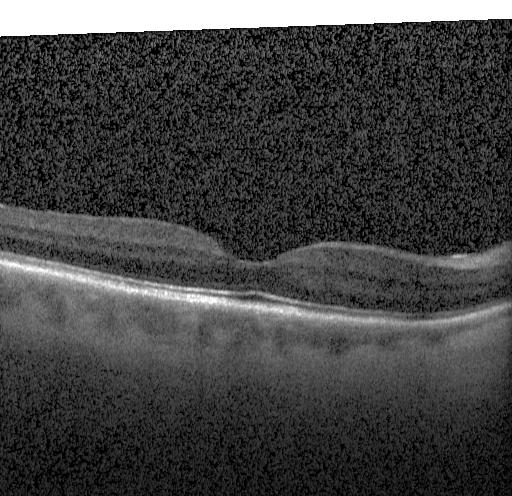

Assessment: neither CNV, DME, nor drusen.